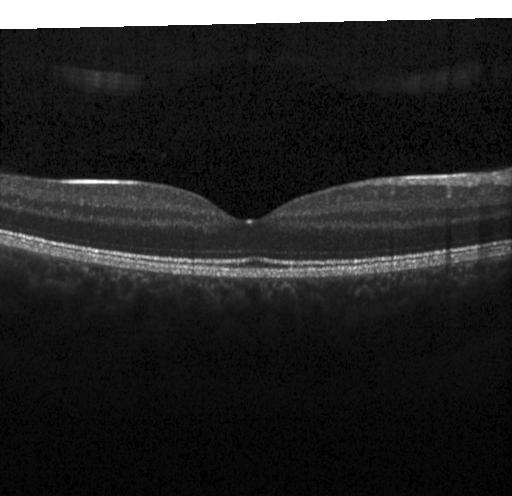
Macular scan, retinal OCT cross-section
Diagnosis: no evidence of choroidal neovascularization, diabetic macular edema, or drusen.